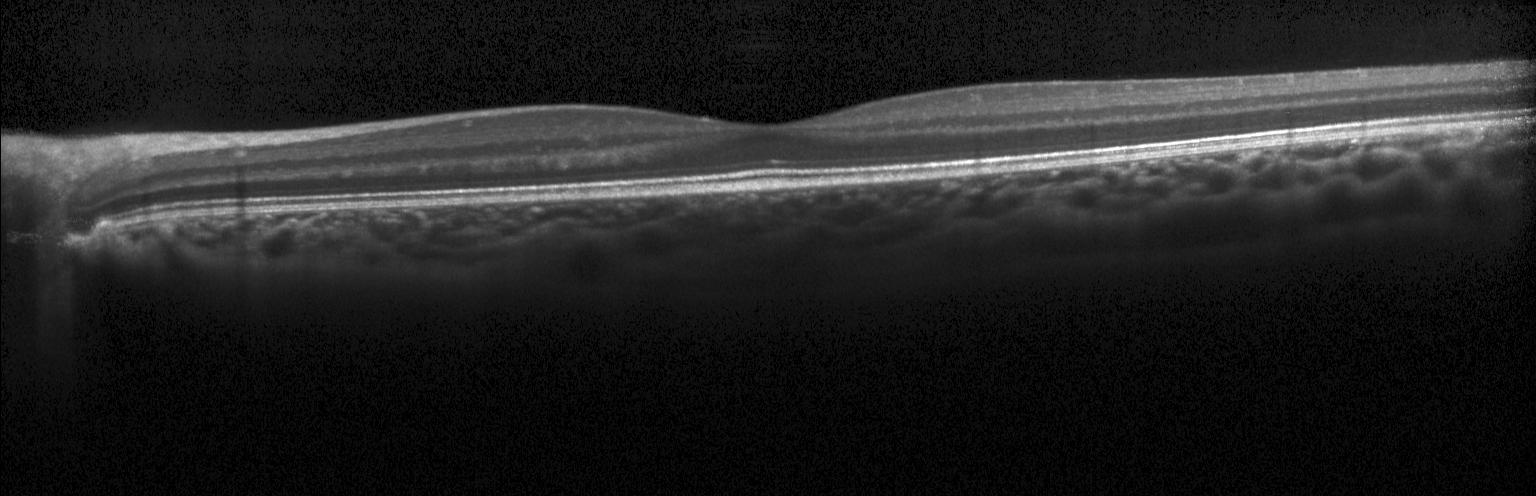 OCT line scan.
Finding: no CNV, DME, or drusen.